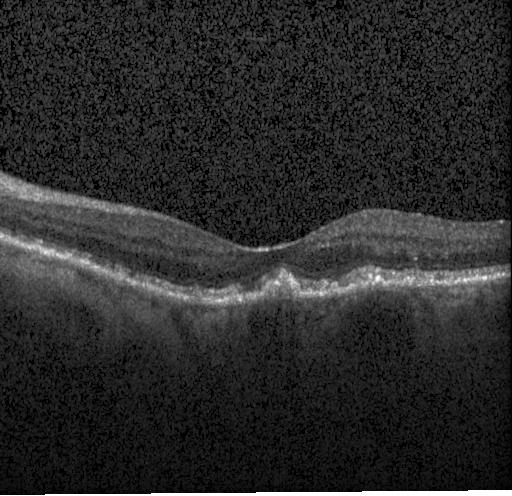
SD-OCT · OCT line scan — The scan shows sub-RPE drusenoid deposits.